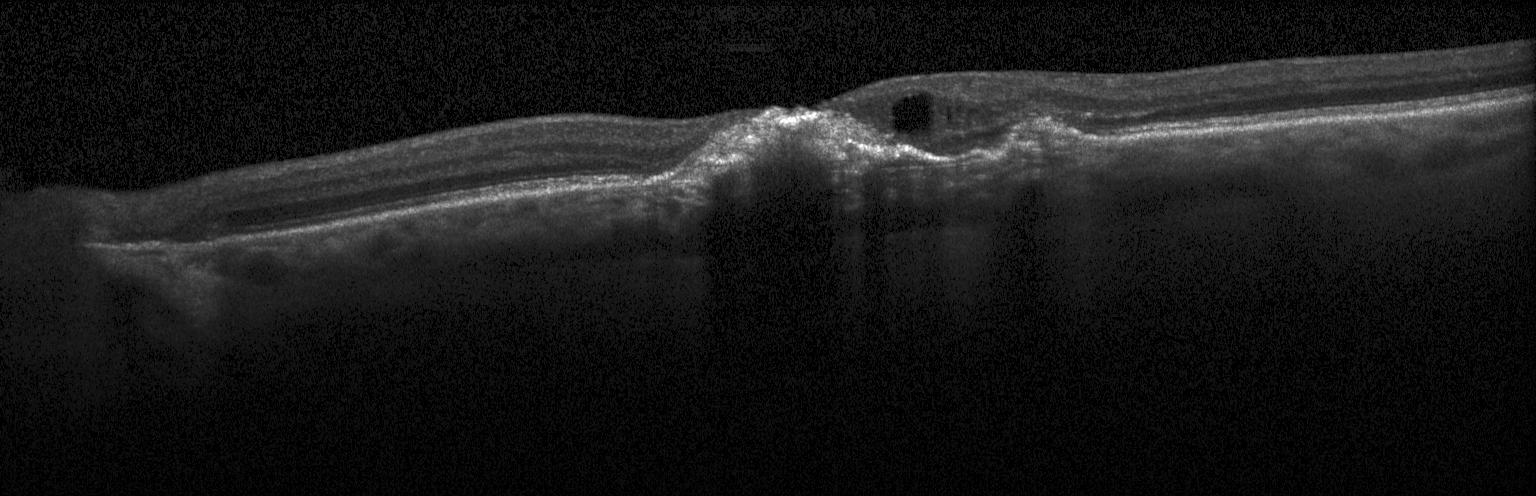 Retinal OCT cross-section · fovea-centered. Dx: choroidal neovascularization (CNV).